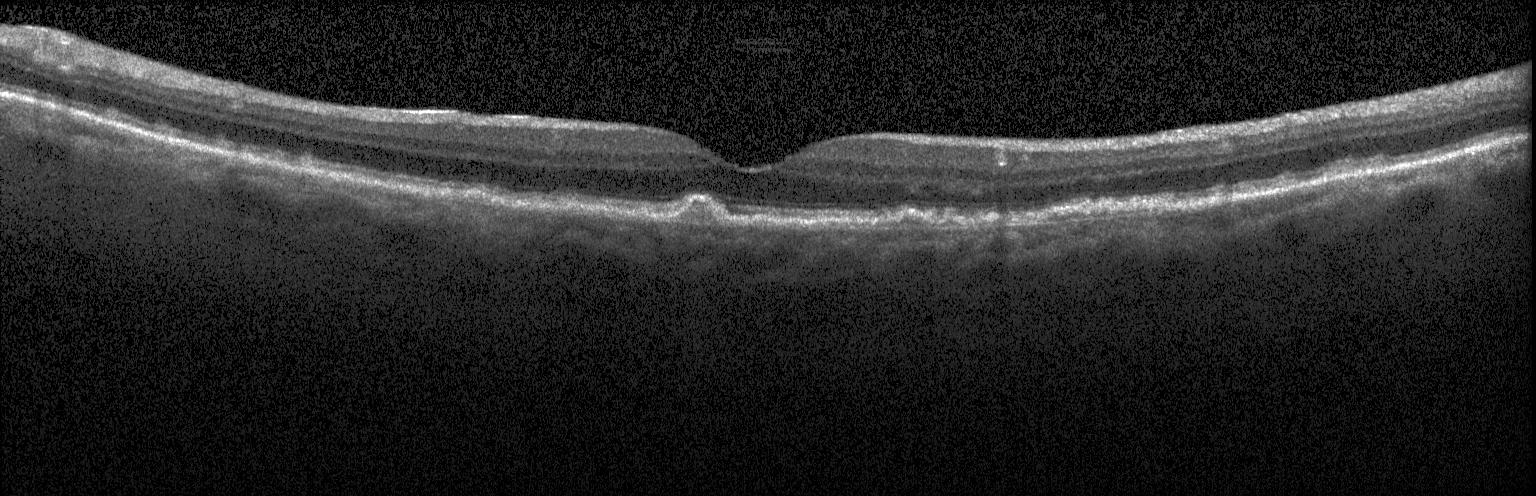
Impression: multiple drusen.